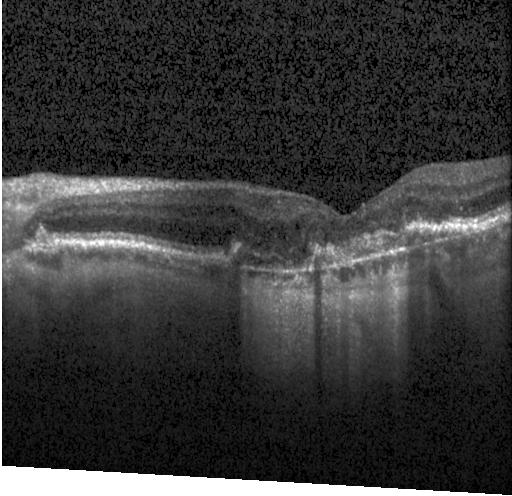
Macular OCT: a choroidal neovascular membrane.